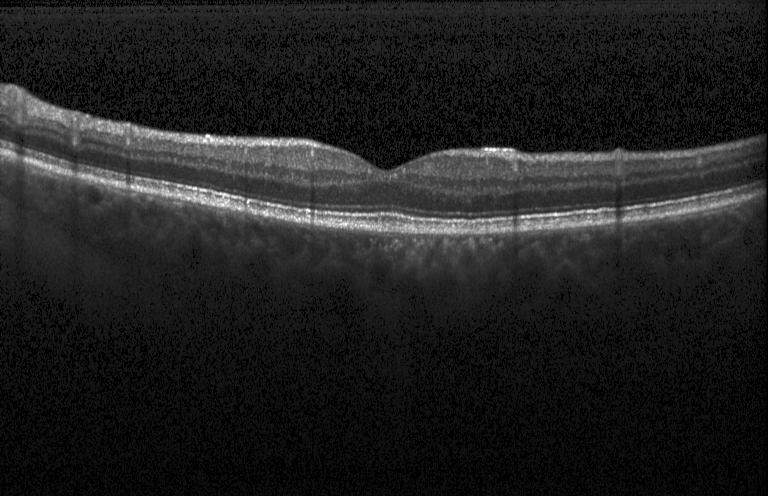

OCT B-scan.
The scan shows no choroidal neovascularization, no diabetic macular edema, and no drusen.